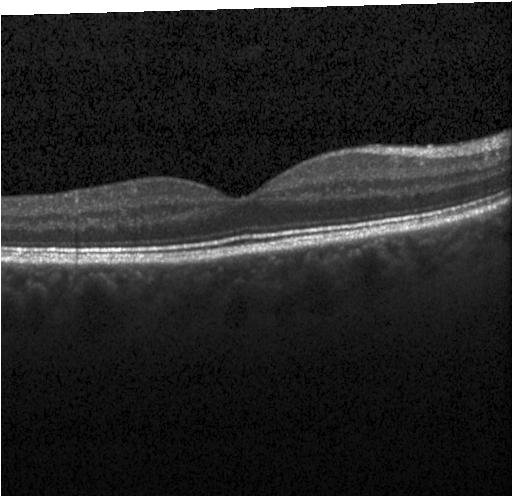 OCT line scan · Heidelberg Spectralis OCT system · horizontal scan through the fovea — Assessment: no choroidal neovascularization, no diabetic macular edema, and no drusen.